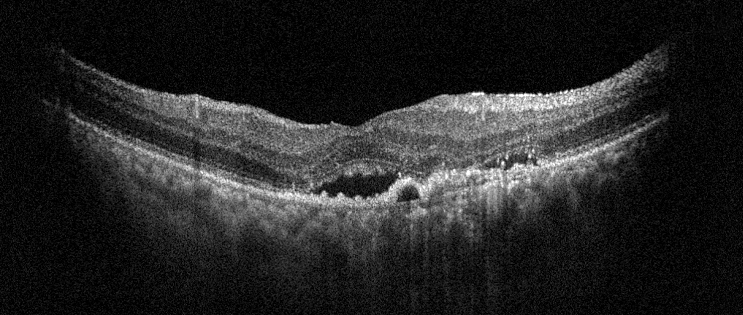 Macular scan; optical coherence tomography B-scan; OD; instrument: Optovue Avanti RTVue XR
Age-related macular degeneration (AMD).